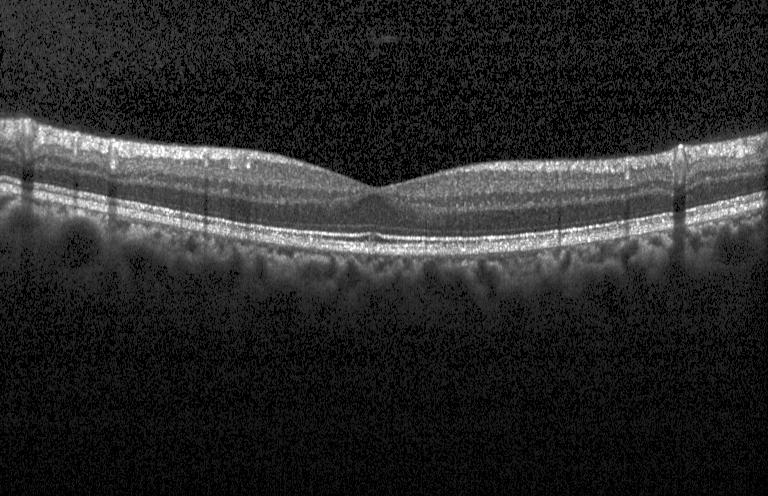 Retinal OCT cross-section, Heidelberg Spectralis, through the macula
Impression: neither CNV, DME, nor drusen.